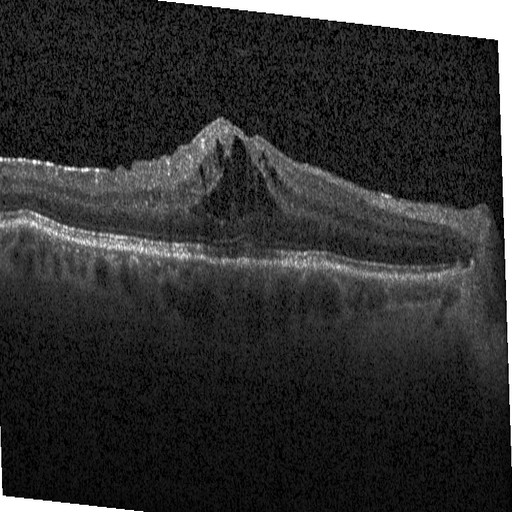

Through the macula, Heidelberg Spectralis OCT system, spectral-domain OCT, OCT line scan
Finding: DME.